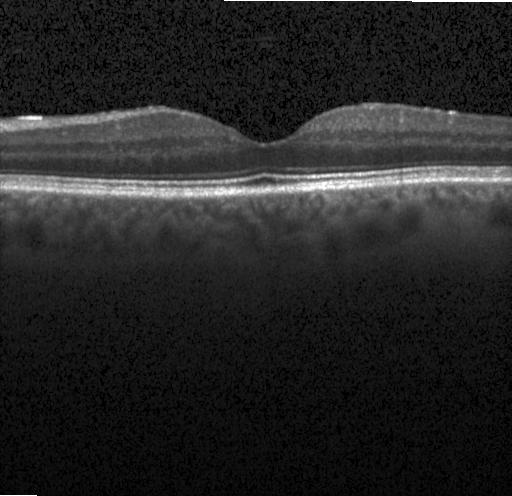

Retinal OCT B-scan; through the macula; acquired on a Heidelberg Spectralis; spectral-domain OCT
Assessment: neither choroidal neovascularization, diabetic macular edema, nor drusen.